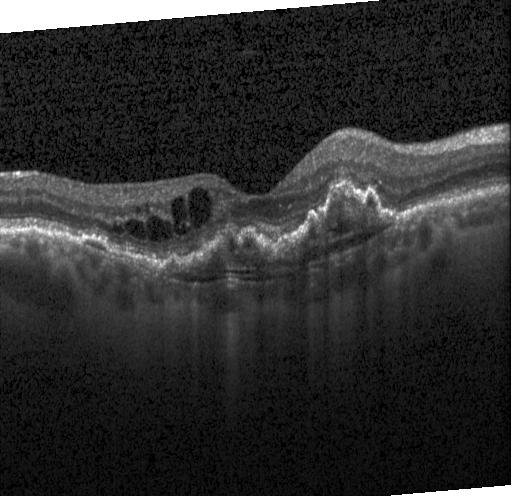

SD-OCT · fovea-centered · retinal OCT cross-section · Heidelberg Spectralis. Diagnosis: a choroidal neovascular membrane.